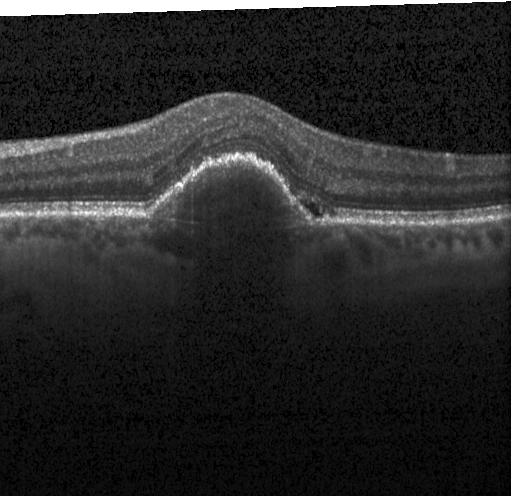
OCT B-scan · through the macula. The scan shows a choroidal neovascular membrane.